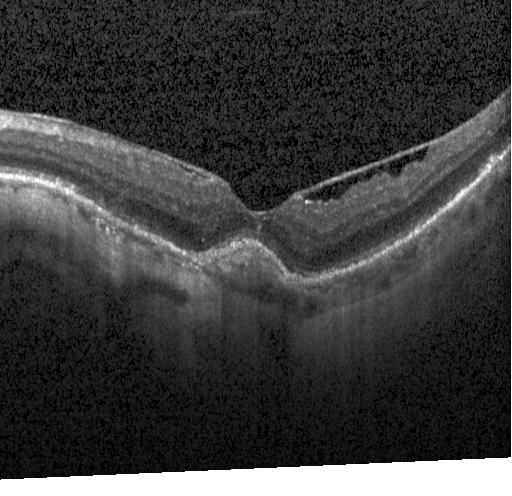
Spectral-domain optical coherence tomography · fovea-centered · OCT B-scan
Impression: choroidal neovascularization.